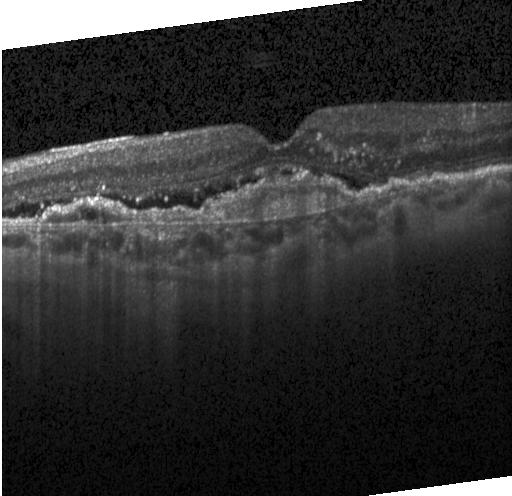

Retinal OCT B-scan, Heidelberg Spectralis, SD-OCT, through the macula. Finding: CNV.